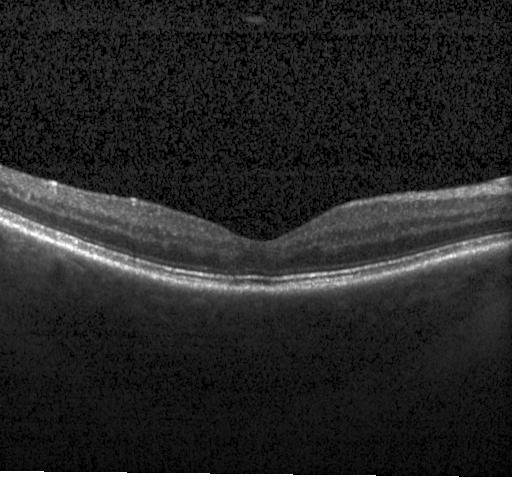 Retinal OCT cross-section showing neither CNV, DME, nor drusen.